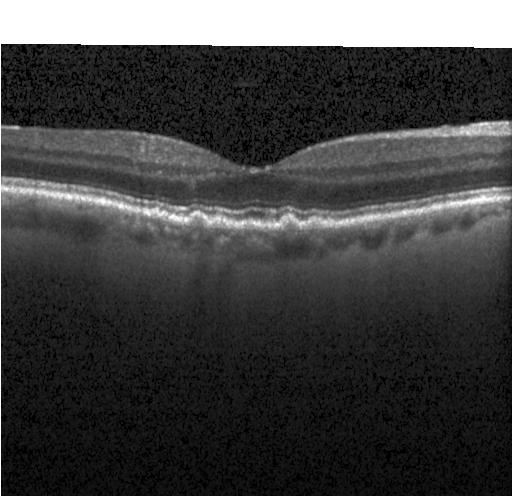 Optical coherence tomography B-scan · Heidelberg Spectralis OCT system. Finding: drusen.